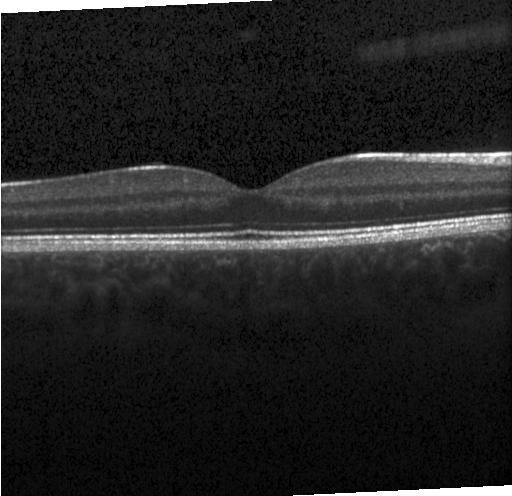

Macular OCT: no evidence of choroidal neovascularization, diabetic macular edema, or drusen.